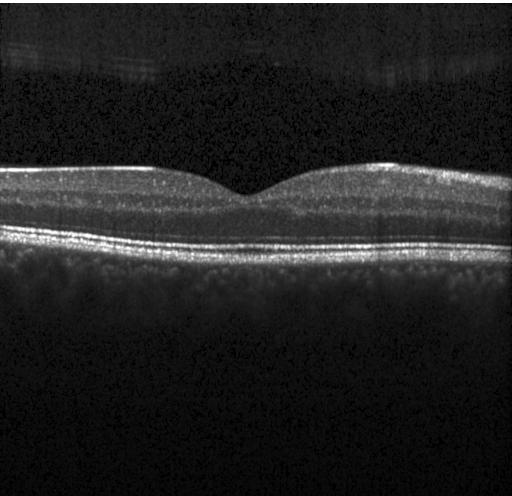

Acquired on a Heidelberg Spectralis; spectral-domain OCT; fovea-centered; OCT line scan — Macular OCT: neither choroidal neovascularization, diabetic macular edema, nor drusen.